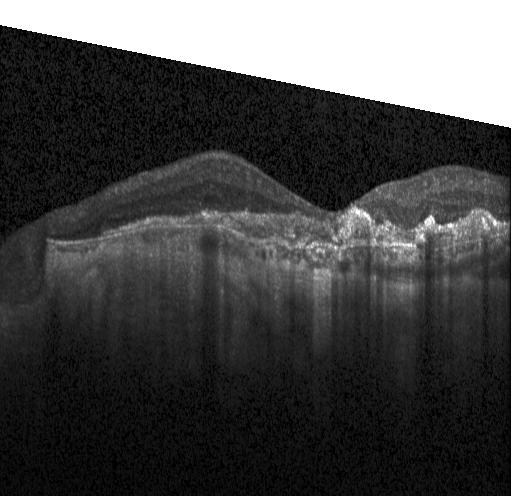 Finding: choroidal neovascularization (CNV).